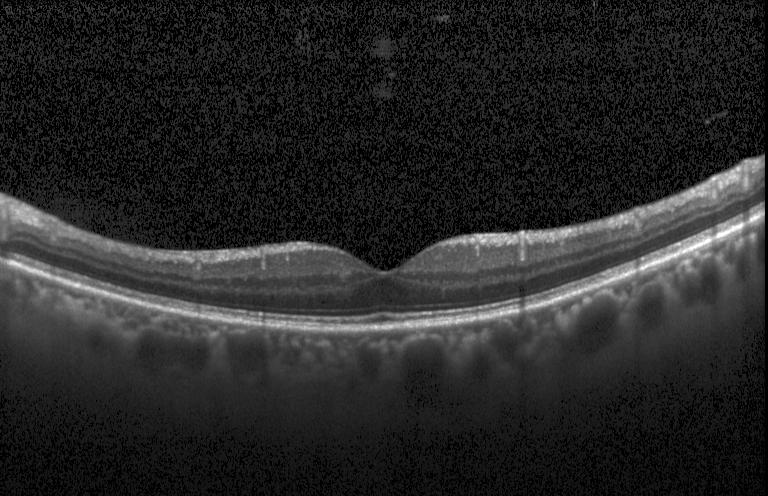
Optical coherence tomography B-scan. Dx: no evidence of CNV, DME, or drusen.